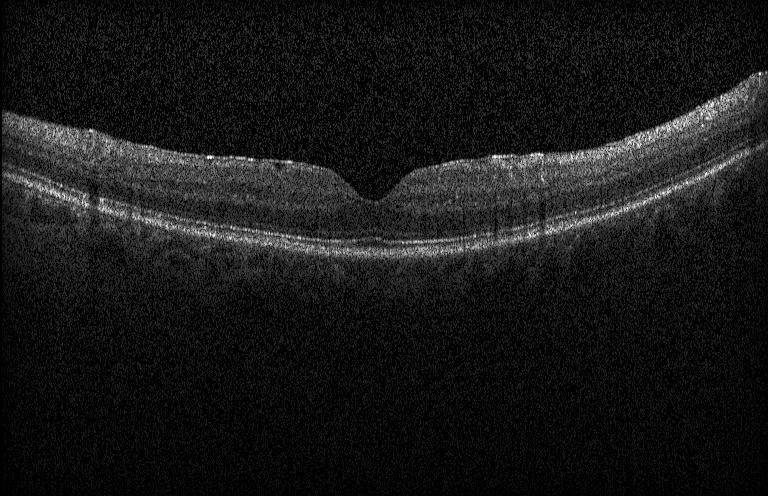
Dx: no CNV, no DME, and no drusen.